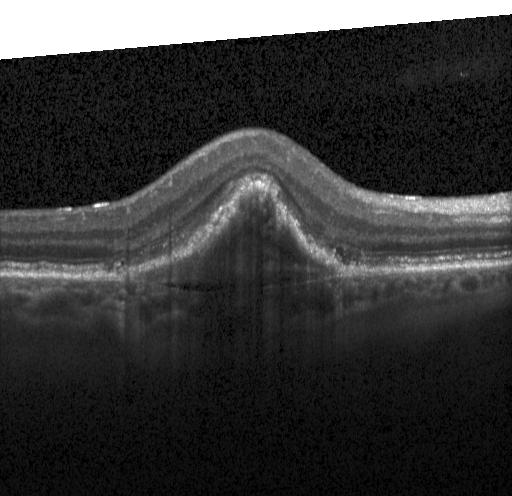
Retinal OCT cross-section
This B-scan demonstrates a choroidal neovascular membrane.